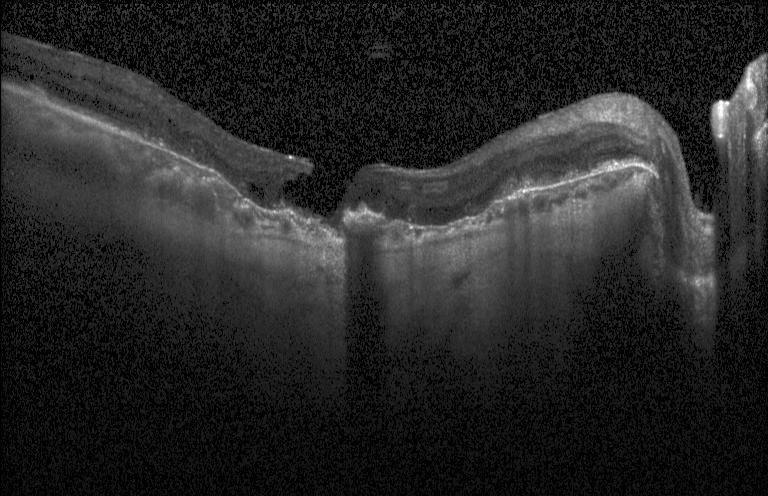

Acquired on a Heidelberg Spectralis. Macular scan. Optical coherence tomography scan. Spectral-domain OCT.
Diagnosis: a choroidal neovascular membrane.